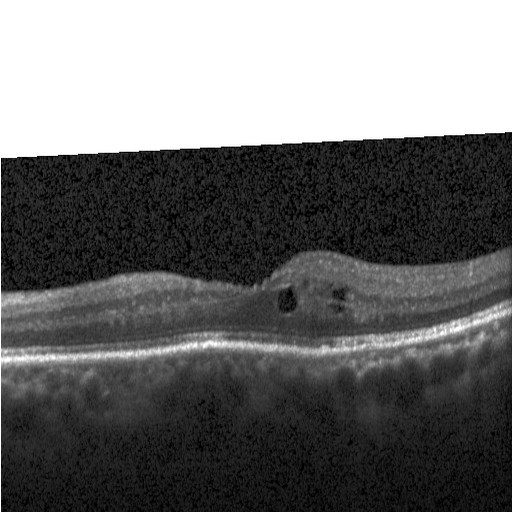

Finding: DME.